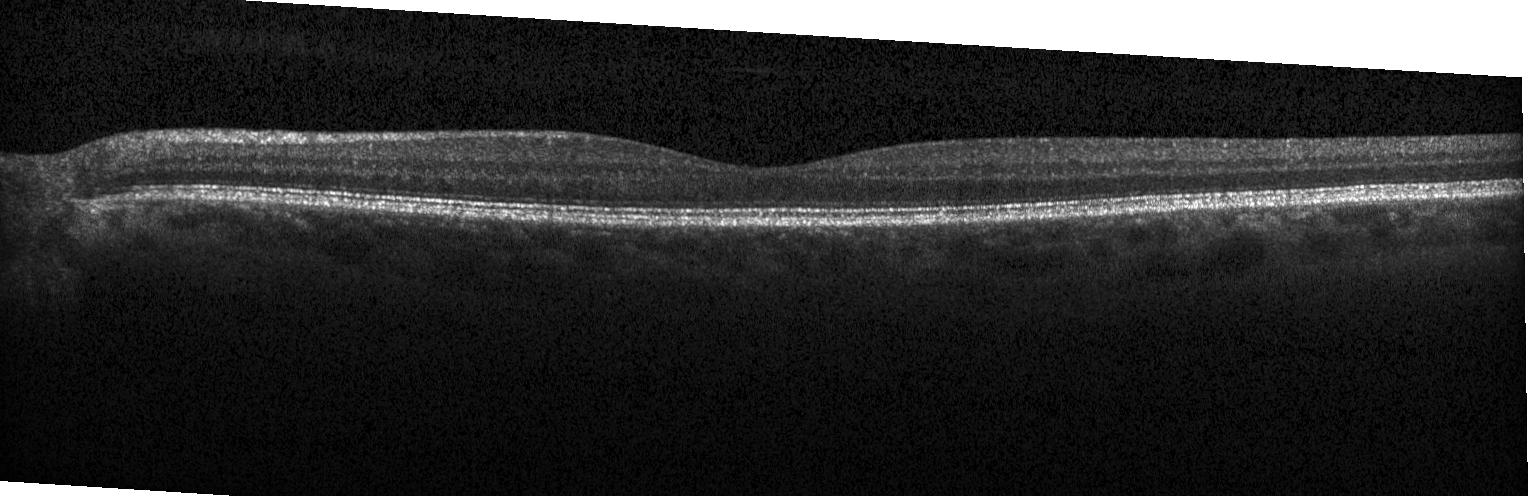

Optical coherence tomography scan; macular scan. Finding: no evidence of choroidal neovascularization, diabetic macular edema, or drusen.